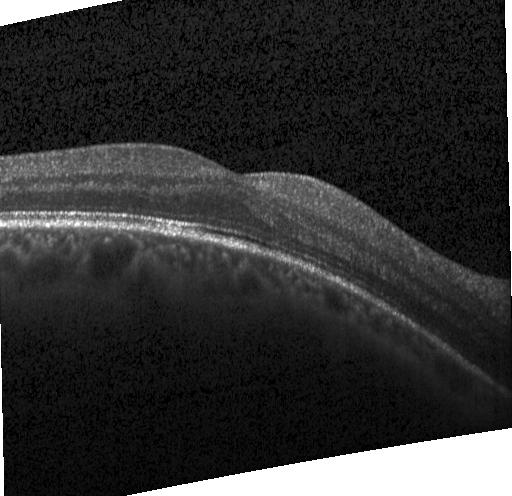
Retinal OCT B-scan · spectral-domain OCT.
The scan shows no evidence of choroidal neovascularization, diabetic macular edema, or drusen.